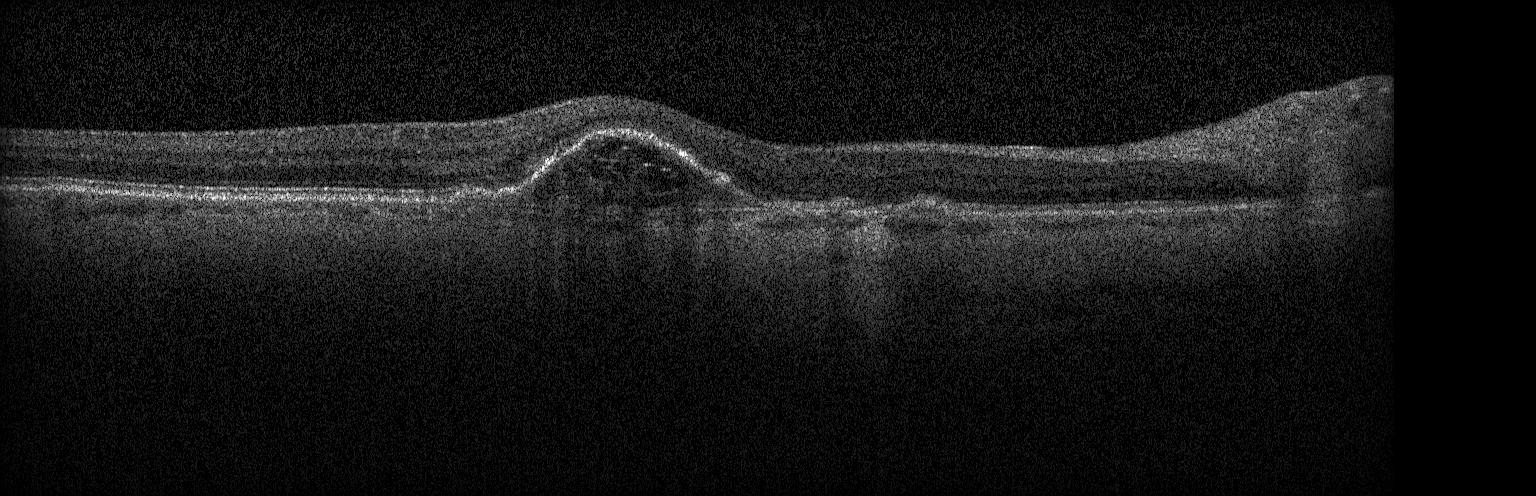

Assessment: a choroidal neovascular membrane.